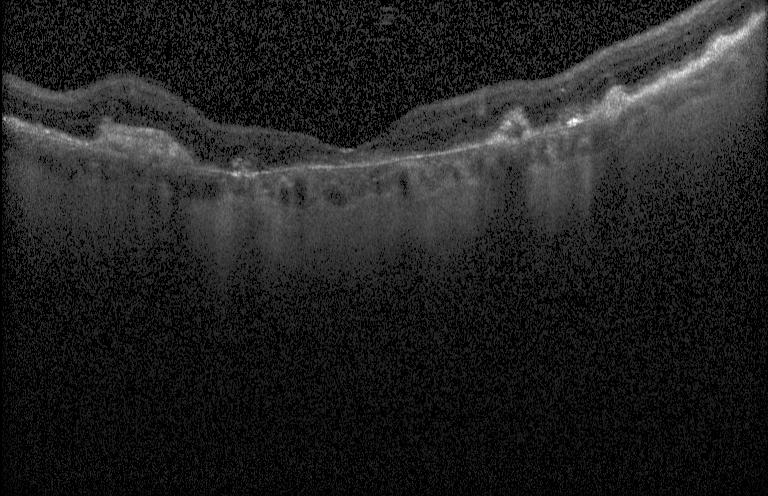 A choroidal neovascular membrane.